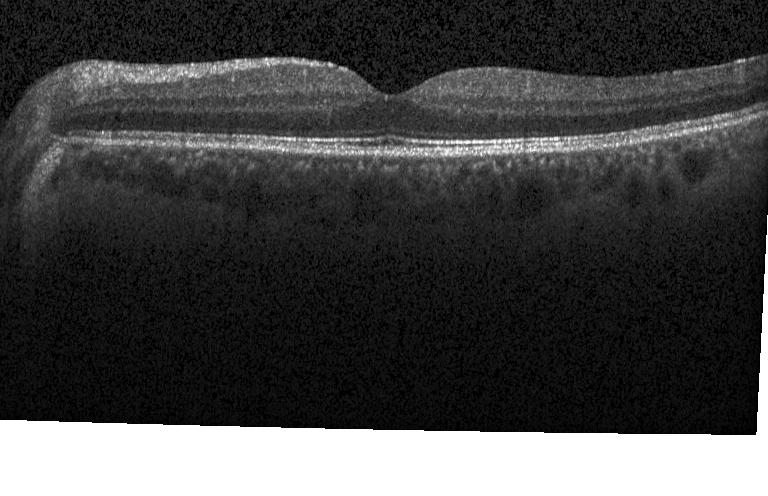 Diagnosis: no evidence of choroidal neovascularization, diabetic macular edema, or drusen.